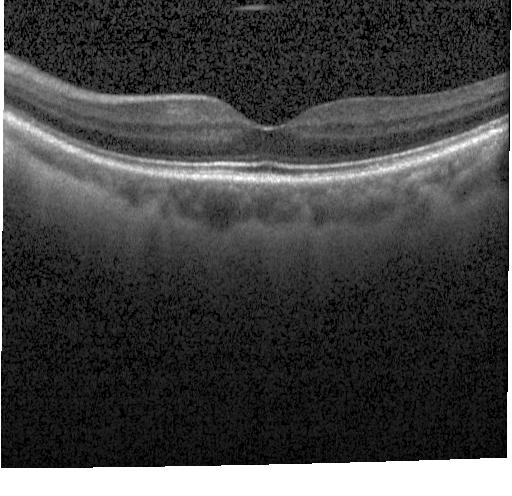
Heidelberg Spectralis · macular scan · OCT line scan.
This B-scan demonstrates no choroidal neovascularization, no diabetic macular edema, and no drusen.